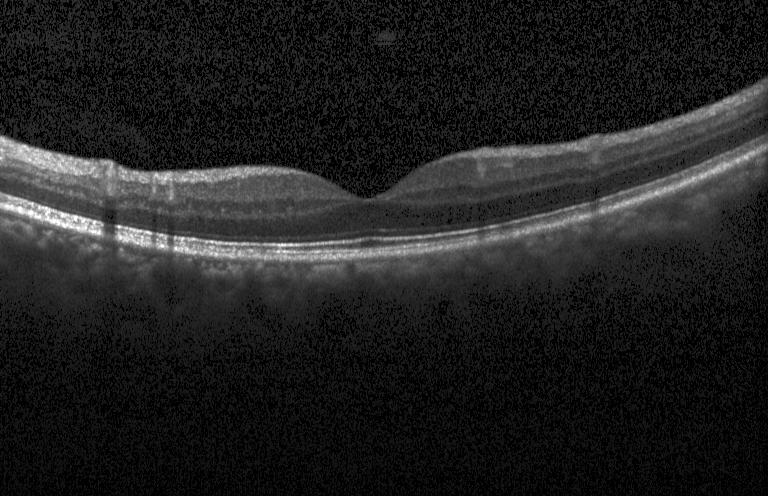 Acquired on a Heidelberg Spectralis, OCT B-scan, spectral-domain OCT, centered on the fovea — This B-scan demonstrates no evidence of choroidal neovascularization, diabetic macular edema, or drusen.